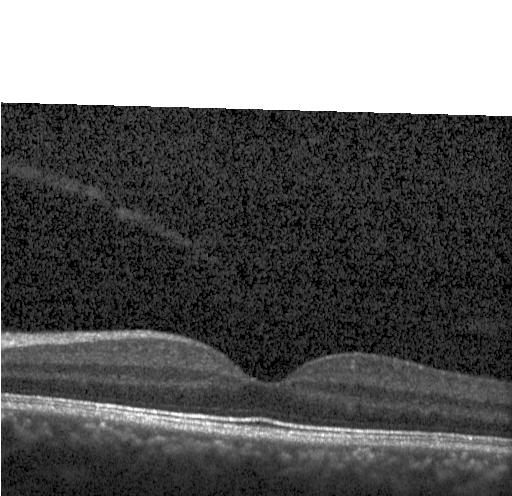
Diagnosis: neither choroidal neovascularization, diabetic macular edema, nor drusen.